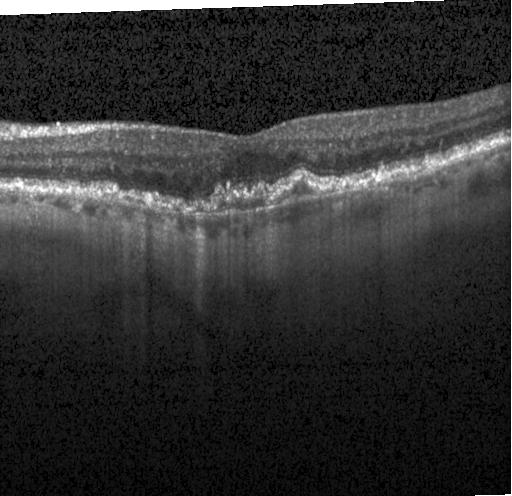 Retinal OCT B-scan, spectral-domain optical coherence tomography — OCT finding: a choroidal neovascular membrane.